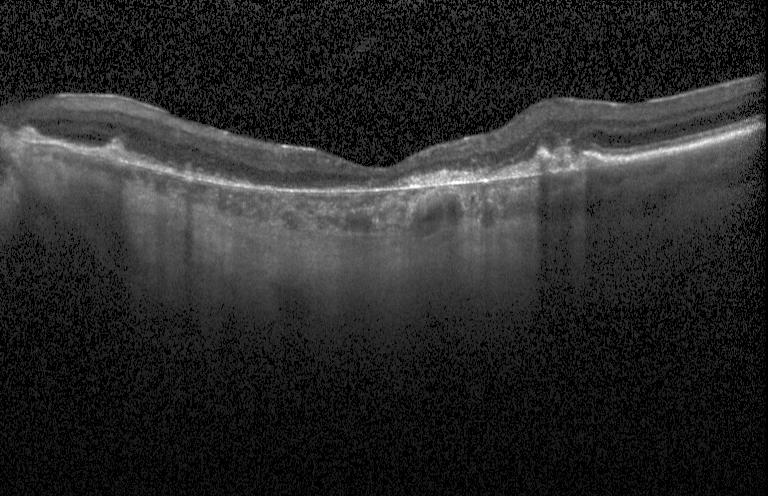
Retinal OCT B-scan; macular scan; acquired on a Heidelberg Spectralis; SD-OCT
Dx: CNV.